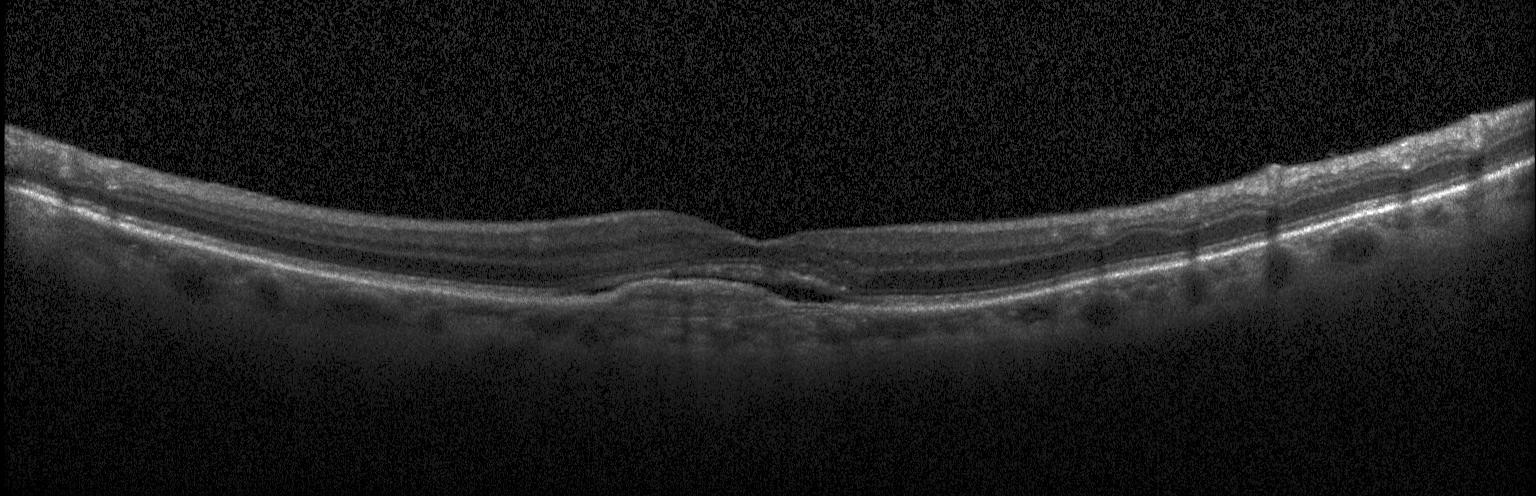

Macular OCT demonstrating a choroidal neovascular membrane.